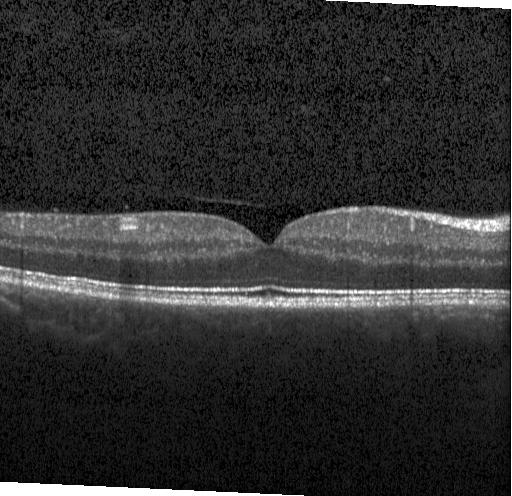 Retinal OCT cross-section. Spectral-domain OCT
Impression: no evidence of choroidal neovascularization, diabetic macular edema, or drusen.